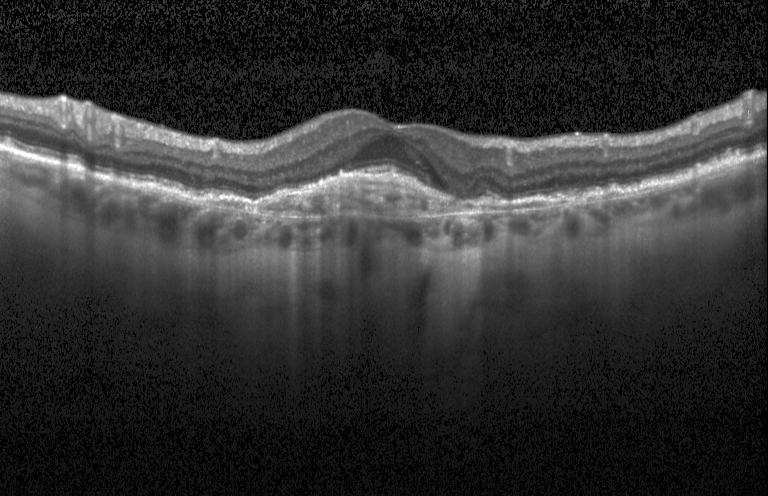

Optical coherence tomography scan, Heidelberg Spectralis OCT system
Finding: a choroidal neovascular membrane.